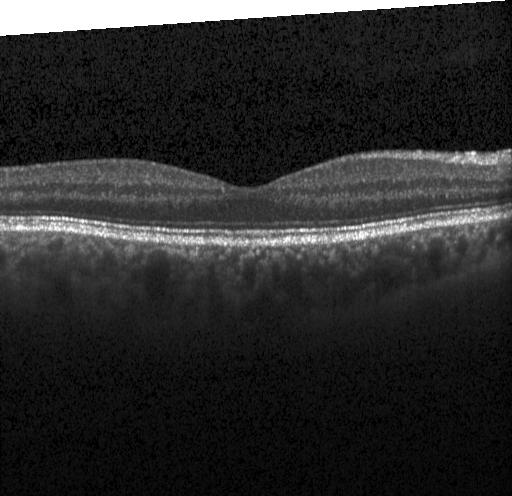

Spectral-domain optical coherence tomography · optical coherence tomography B-scan · macular scan — Impression: no choroidal neovascularization, diabetic macular edema, or drusen.